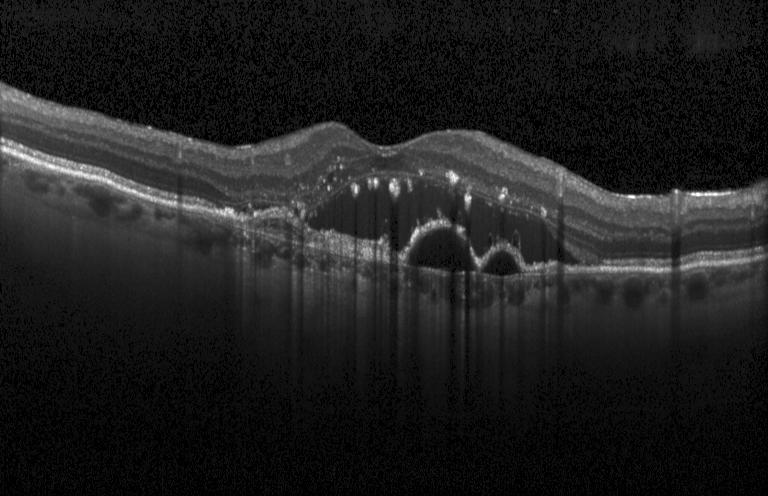

Dx: a choroidal neovascular membrane.